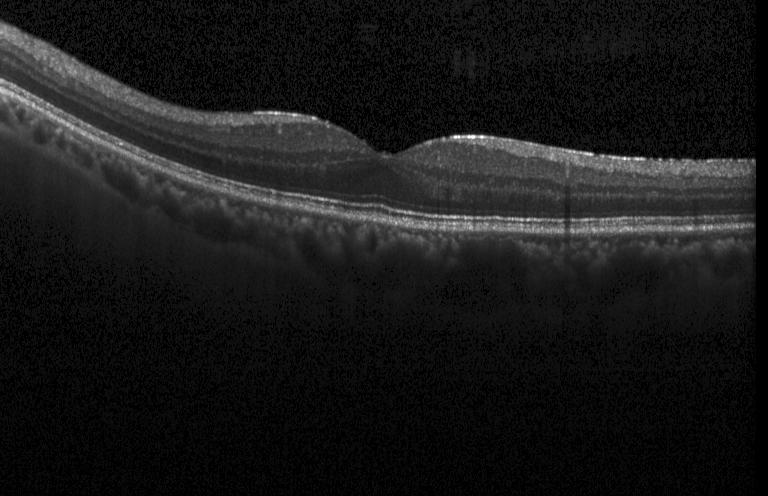 SD-OCT, retinal OCT B-scan, Heidelberg Spectralis OCT system. Diagnosis: no evidence of CNV, DME, or drusen.